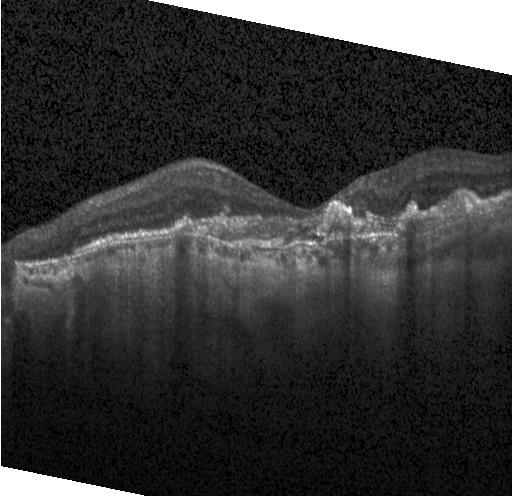

Assessment: choroidal neovascularization.